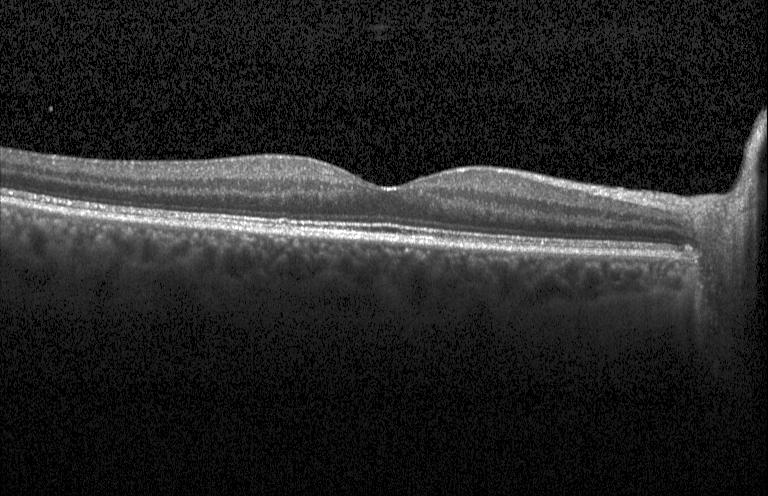
Diagnosis: no CNV, no DME, and no drusen.